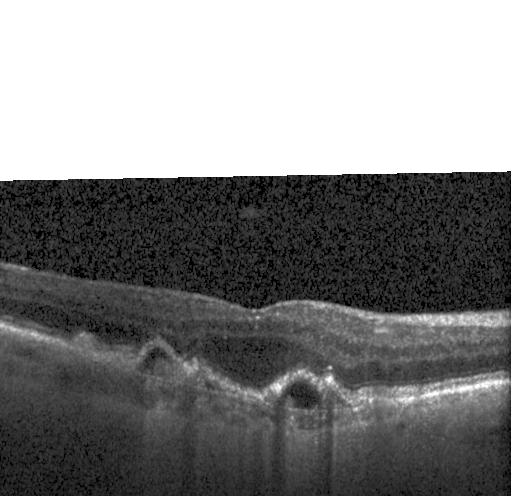

Retinal OCT cross-section, fovea-centered, Heidelberg Spectralis OCT system, SD-OCT
This B-scan demonstrates choroidal neovascularization (CNV).